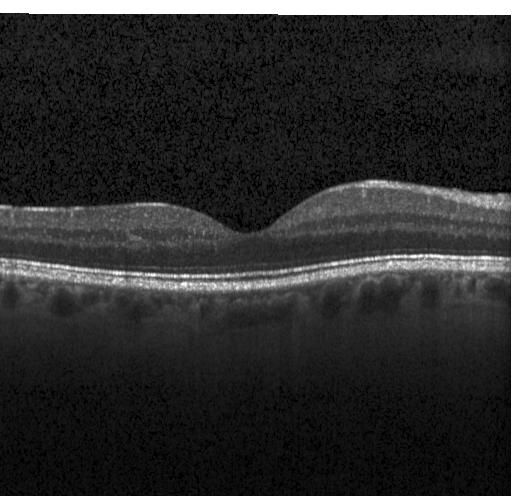 Spectral-domain OCT · Heidelberg Spectralis OCT system · optical coherence tomography scan — Dx: neither choroidal neovascularization, diabetic macular edema, nor drusen.